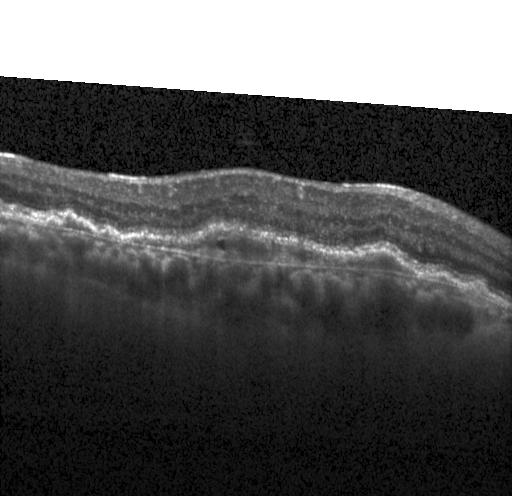
Impression: CNV.